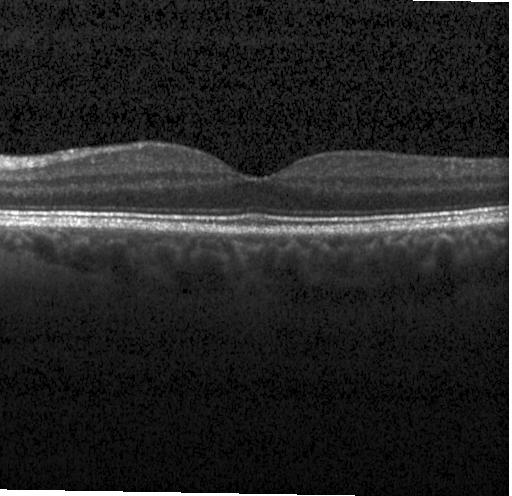 Spectral-domain OCT; Heidelberg Spectralis OCT system; horizontal scan through the fovea; optical coherence tomography B-scan
Macular OCT: no evidence of CNV, DME, or drusen.